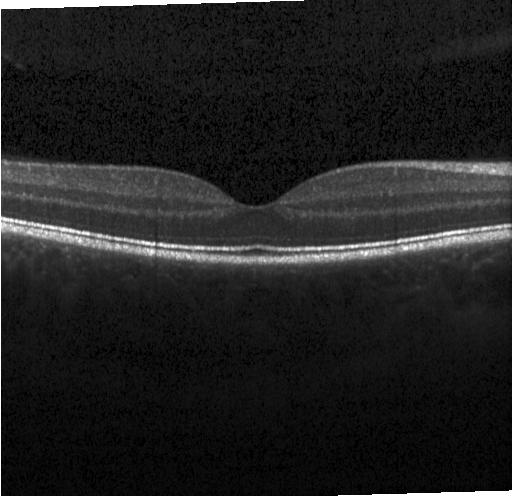 Macular scan · OCT B-scan · SD-OCT · Heidelberg Spectralis OCT system
Finding: no CNV, DME, or drusen.